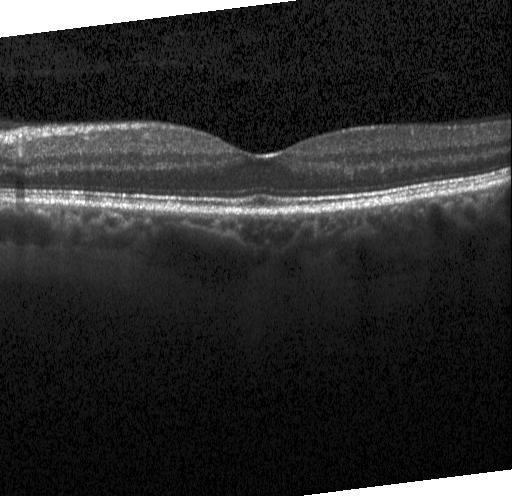

Optical coherence tomography scan.
The scan shows no choroidal neovascularization, diabetic macular edema, or drusen.